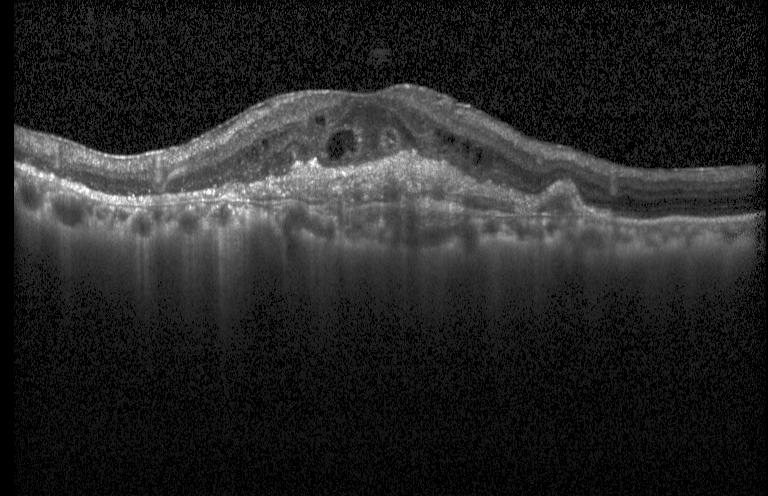 Heidelberg Spectralis OCT system; optical coherence tomography B-scan.
Assessment: a choroidal neovascular membrane.